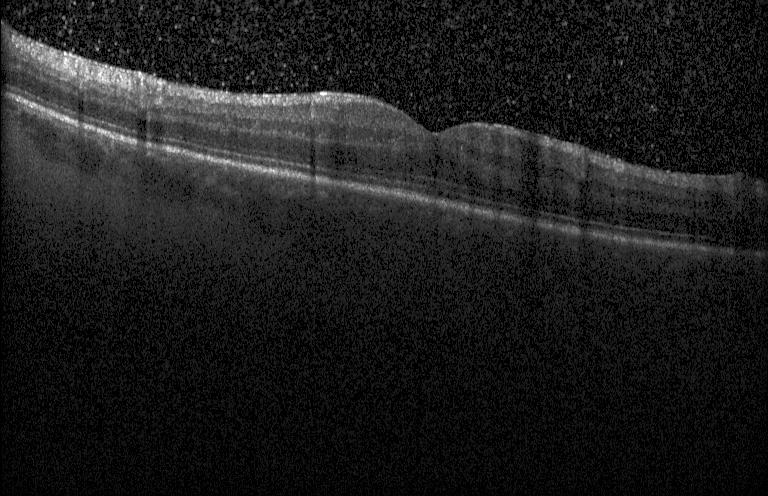
Diagnosis: no evidence of choroidal neovascularization, diabetic macular edema, or drusen.